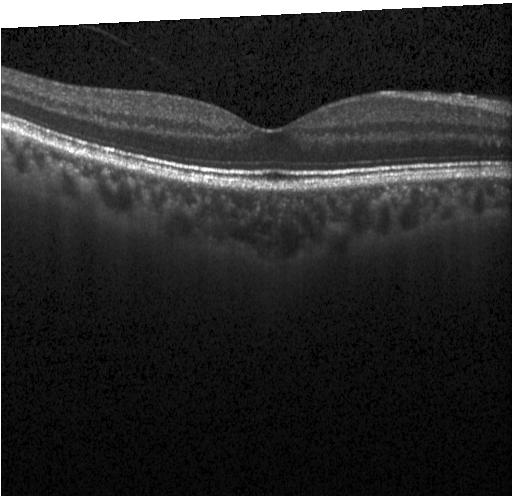
Retinal OCT cross-section — Finding: neither choroidal neovascularization, diabetic macular edema, nor drusen.